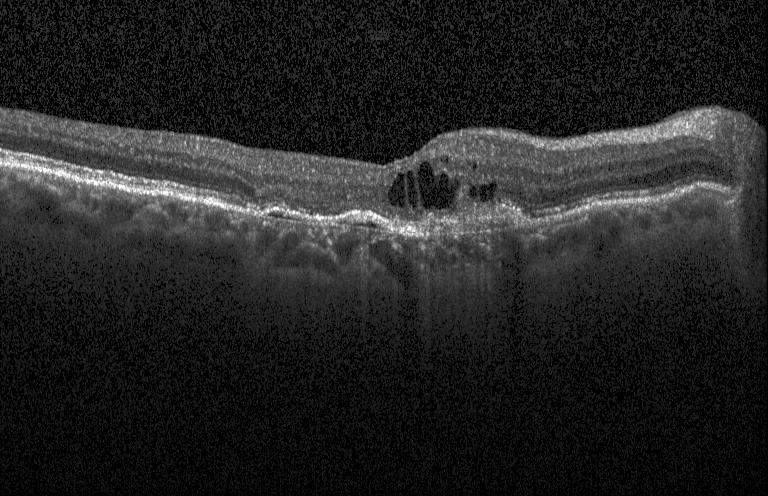
Assessment: a choroidal neovascular membrane.